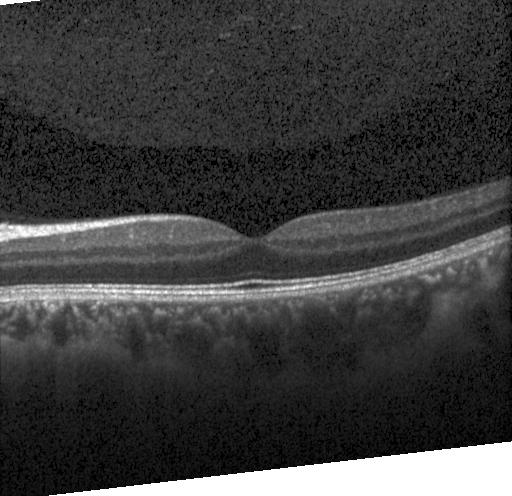 OCT B-scan. The scan shows neither choroidal neovascularization, diabetic macular edema, nor drusen.